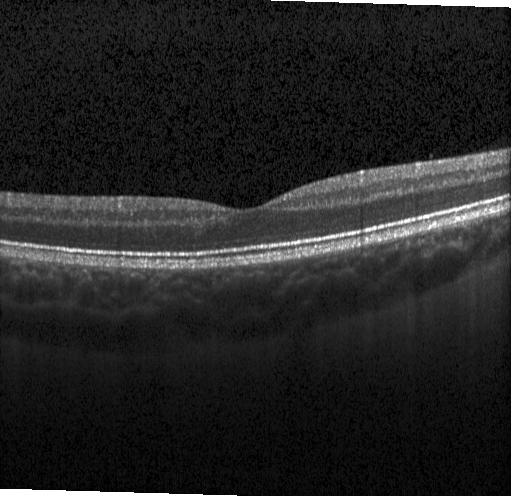
Finding: no choroidal neovascularization, diabetic macular edema, or drusen.